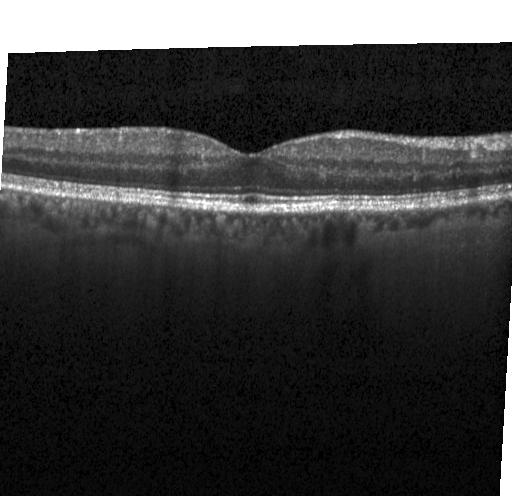

Retinal OCT cross-section; Heidelberg Spectralis — Finding: neither CNV, DME, nor drusen.